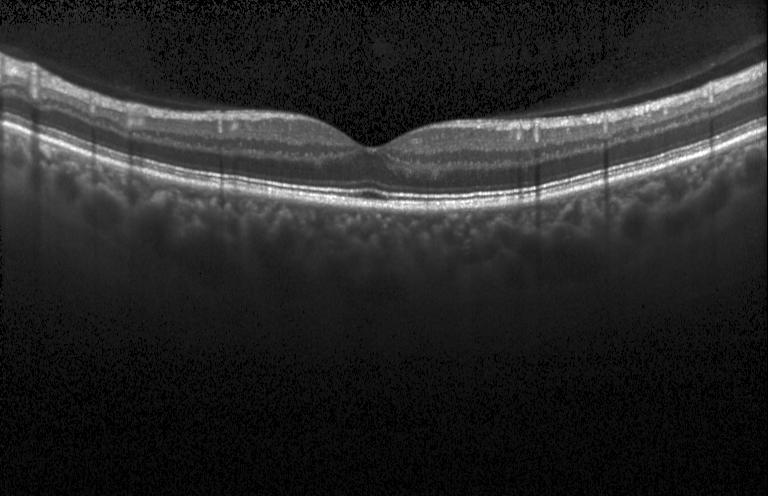

OCT B-scan — Dx: neither choroidal neovascularization, diabetic macular edema, nor drusen.